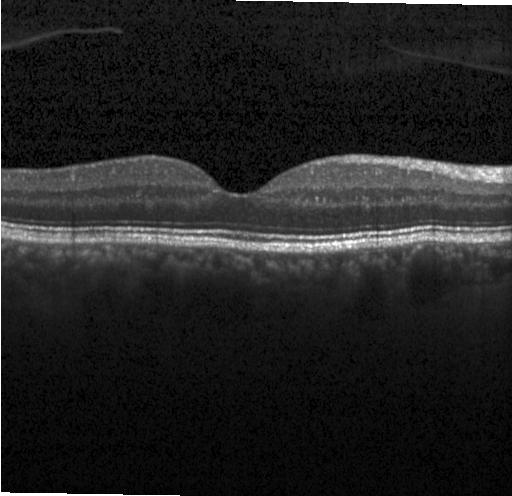

Optical coherence tomography scan, SD-OCT.
Impression: no evidence of choroidal neovascularization, diabetic macular edema, or drusen.